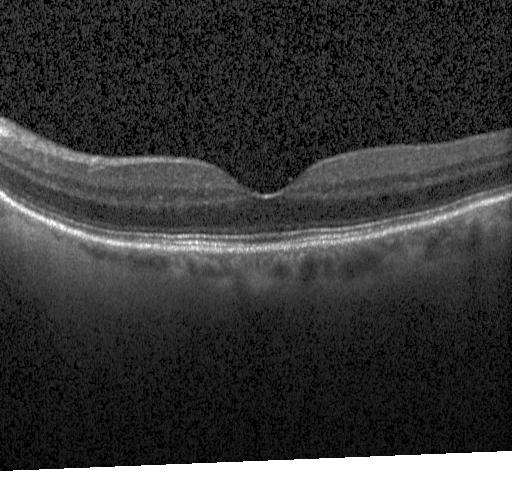
OCT B-scan. Heidelberg Spectralis OCT system — Finding: neither CNV, DME, nor drusen.